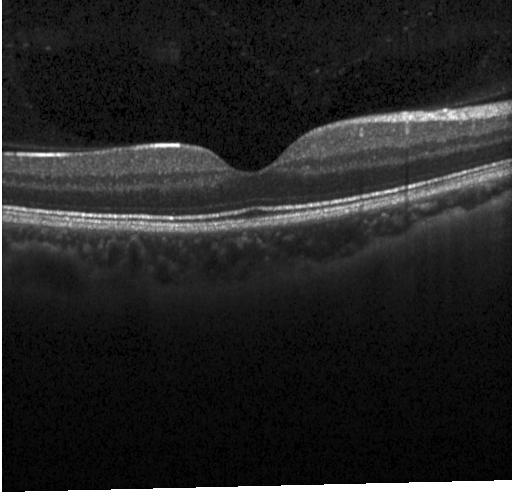 Macular OCT demonstrating no choroidal neovascularization, no diabetic macular edema, and no drusen.